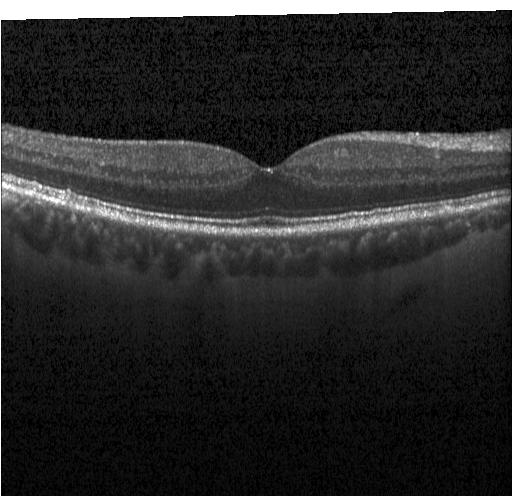 Diagnosis: no CNV, DME, or drusen.